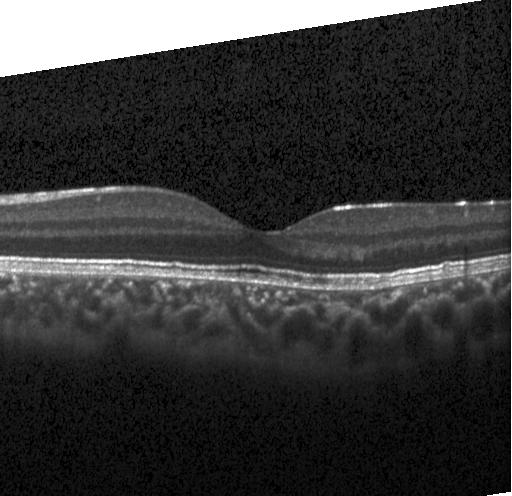

Spectral-domain optical coherence tomography · OCT B-scan · Heidelberg Spectralis. Dx: neither choroidal neovascularization, diabetic macular edema, nor drusen.